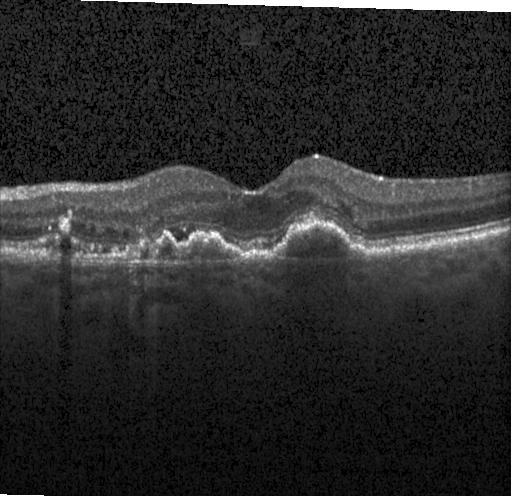
OCT scan showing a choroidal neovascular membrane.